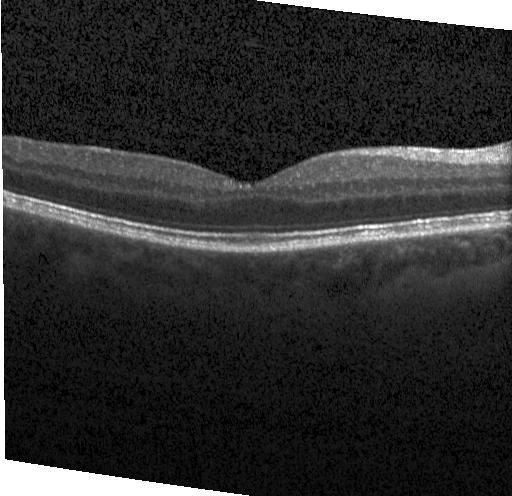 Horizontal scan through the fovea; OCT B-scan; spectral-domain OCT — This B-scan demonstrates neither choroidal neovascularization, diabetic macular edema, nor drusen.